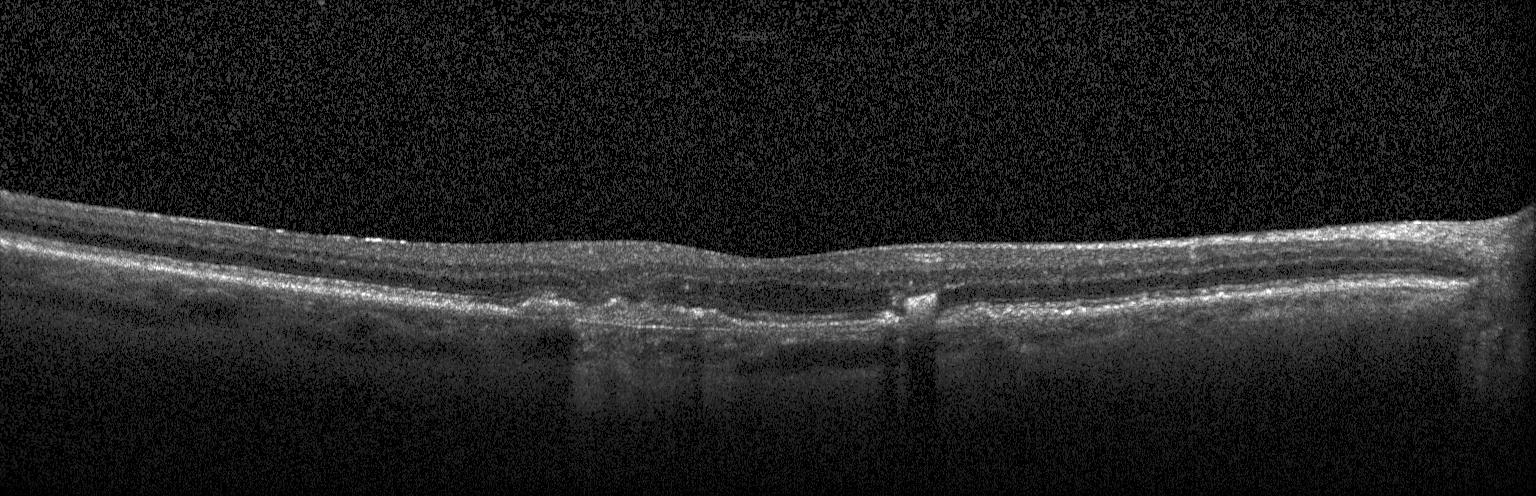

Macular scan, retinal OCT B-scan, Heidelberg Spectralis OCT system
Finding: choroidal neovascularization (CNV).